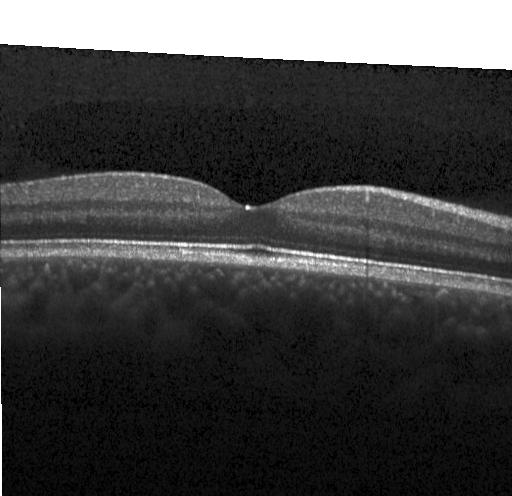

Impression: no CNV, no DME, and no drusen.